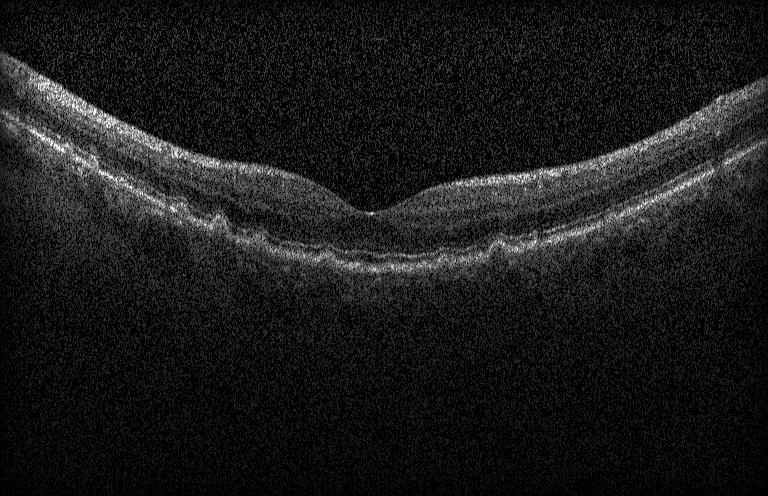 OCT B-scan — Finding: multiple drusen.